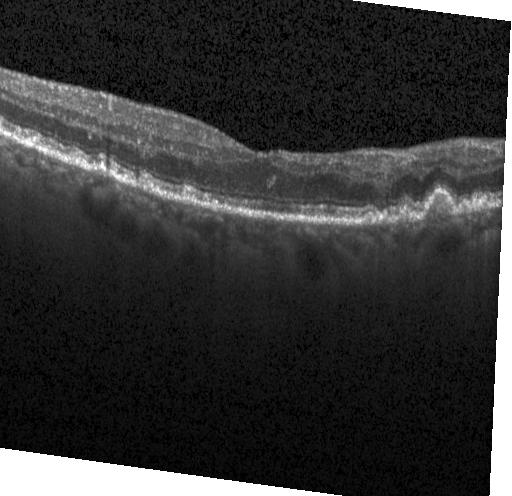
Diagnosis: sub-RPE drusenoid deposits.